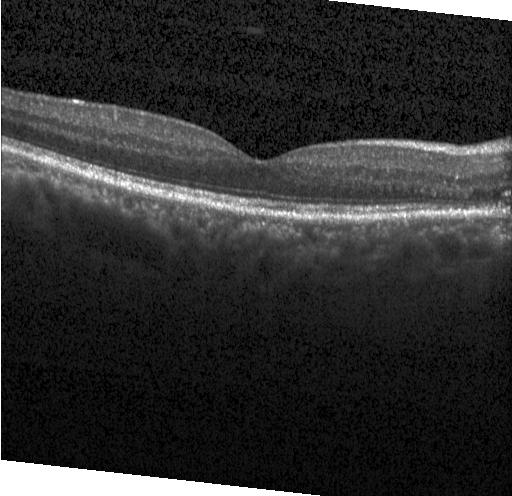

Acquired on a Heidelberg Spectralis, retinal OCT cross-section.
No evidence of CNV, DME, or drusen.